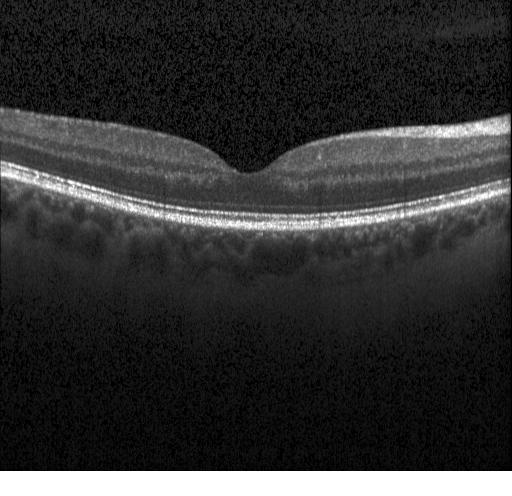
Optical coherence tomography B-scan — This B-scan demonstrates no choroidal neovascularization, no diabetic macular edema, and no drusen.